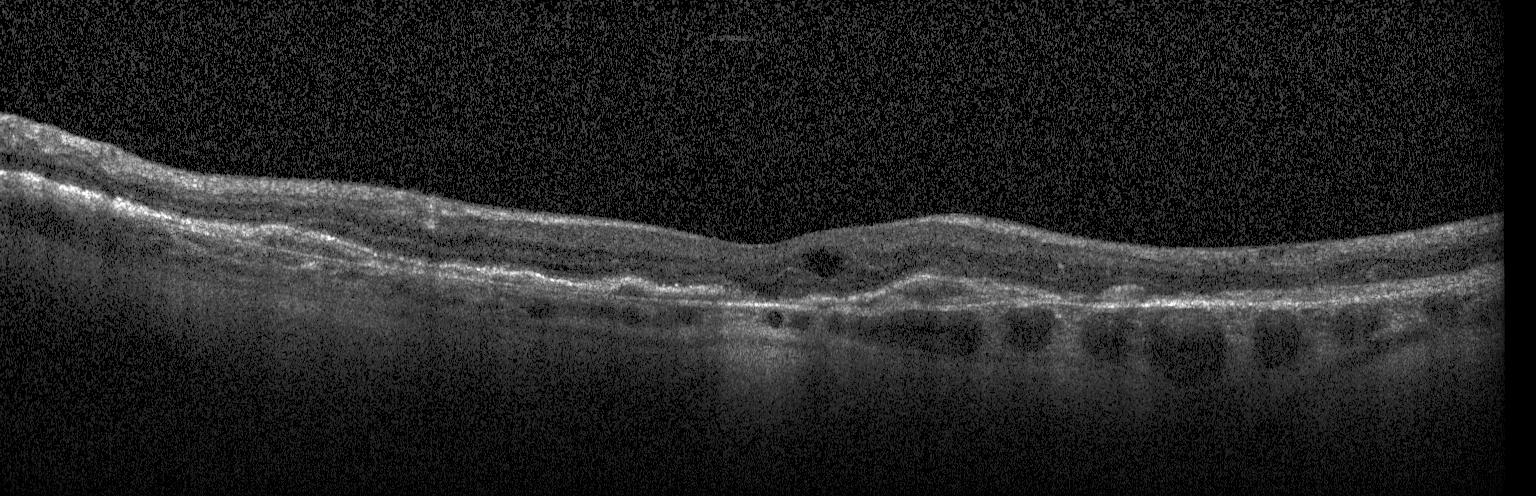

Retinal OCT cross-section.
Macular OCT: a choroidal neovascular membrane.